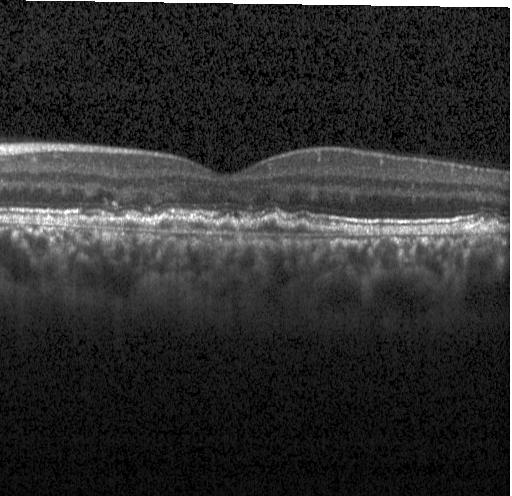
Through the macula · optical coherence tomography B-scan. Finding: a choroidal neovascular membrane.